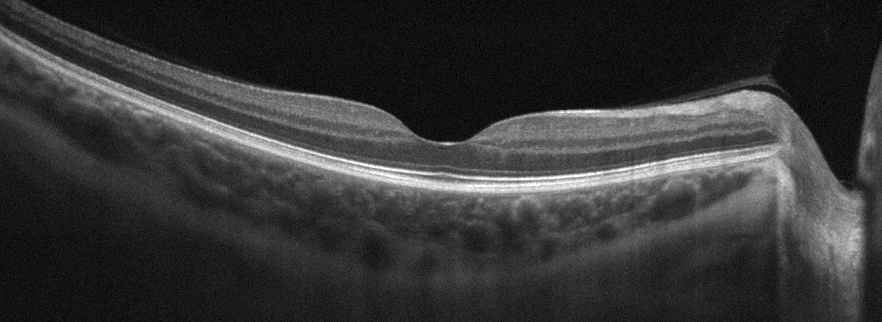

Oculus dexter · OCT line scan. Impression: no AMD, DME, ERM, RAO, RVO, or VID.